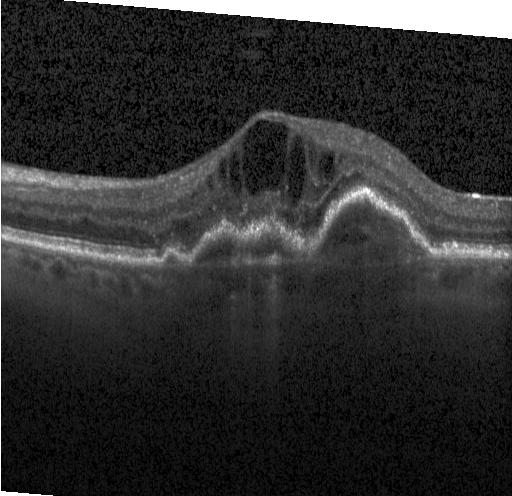
OCT B-scan — Dx: choroidal neovascularization.